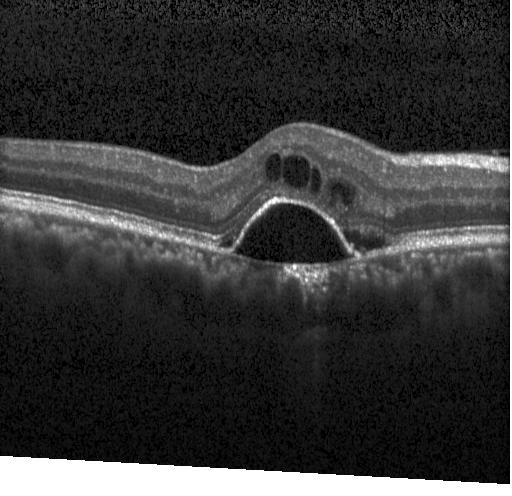 Centered on the fovea, SD-OCT, OCT B-scan
Impression: CNV.